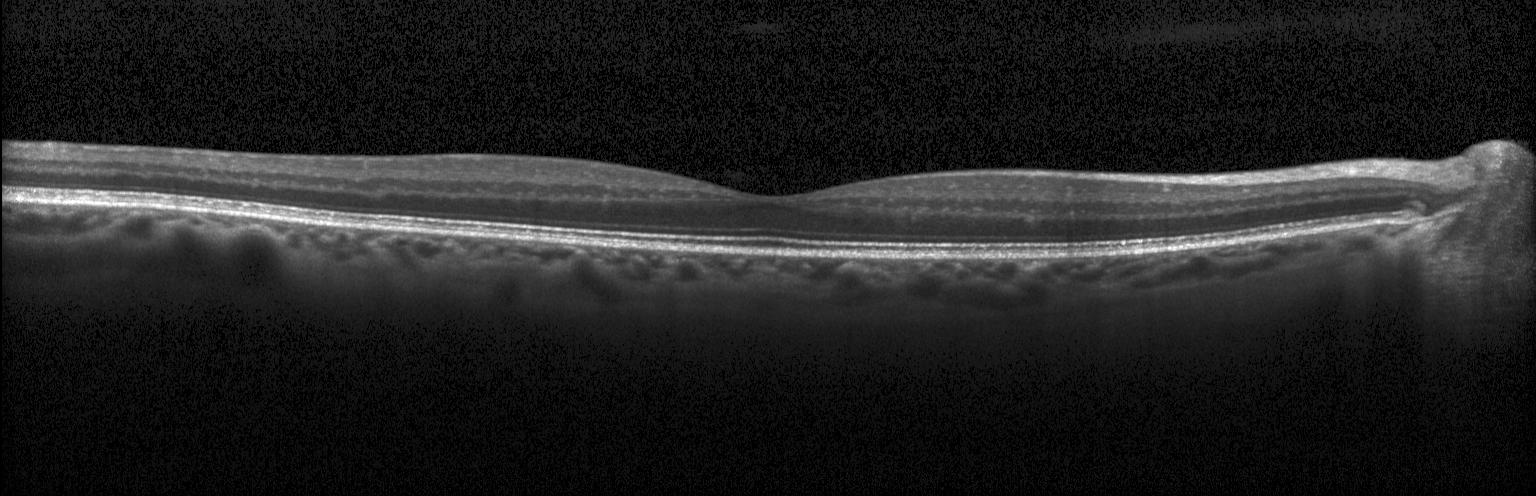

Spectral-domain optical coherence tomography; retinal OCT B-scan; Heidelberg Spectralis OCT system.
Diagnosis: no CNV, DME, or drusen.